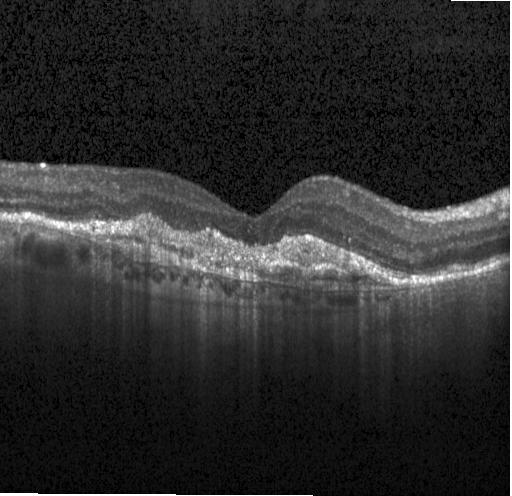 SD-OCT. Retinal OCT cross-section — Assessment: CNV.